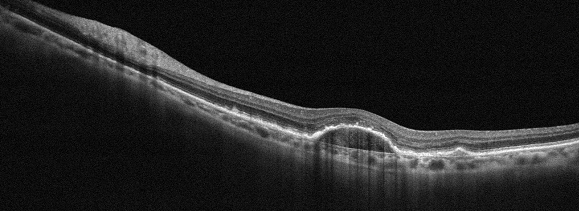
Optovue Avanti RTVue XR; OCT B-scan; macular scan; left eye
Dx: age-related macular degeneration.